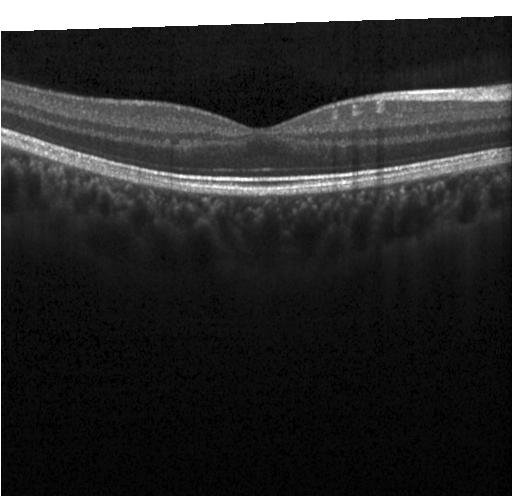 OCT B-scan · acquired on a Heidelberg Spectralis · through the macula. Finding: neither CNV, DME, nor drusen.